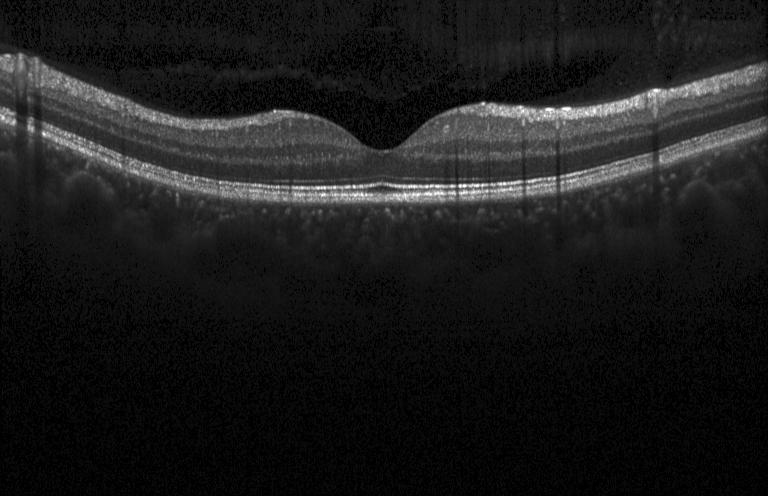

Impression: no evidence of choroidal neovascularization, diabetic macular edema, or drusen.